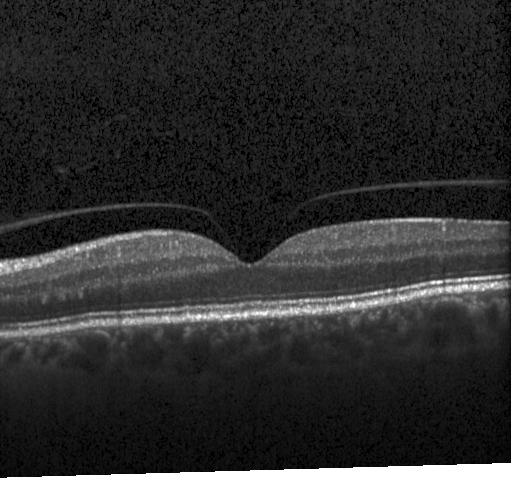

Dx: no CNV, no DME, and no drusen.